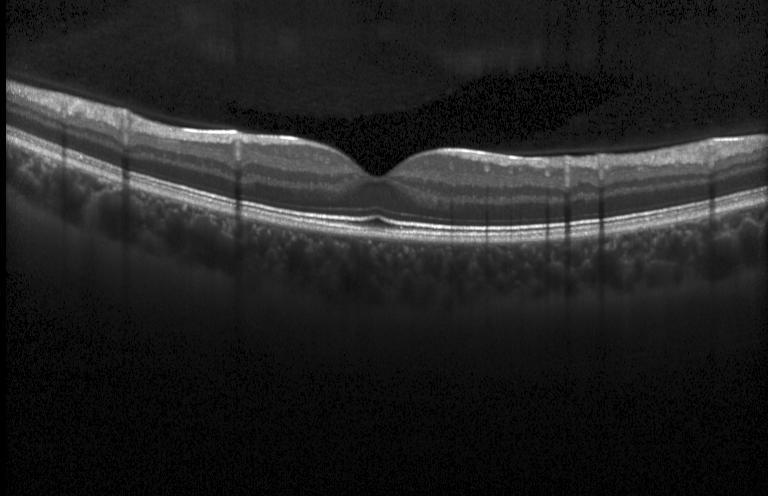 Fovea-centered. Instrument: Heidelberg Spectralis. Spectral-domain OCT. OCT line scan.
Finding: neither choroidal neovascularization, diabetic macular edema, nor drusen.